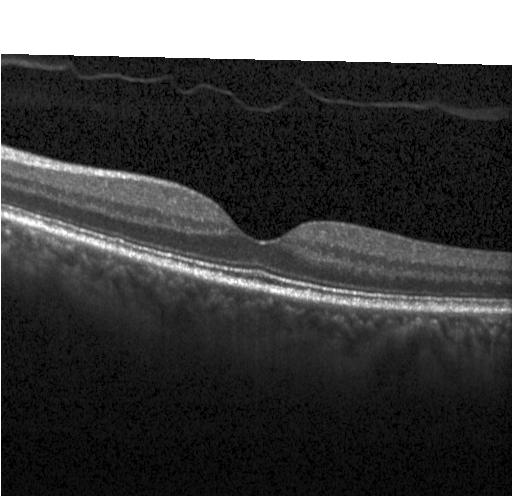 Retinal OCT cross-section showing no evidence of CNV, DME, or drusen.